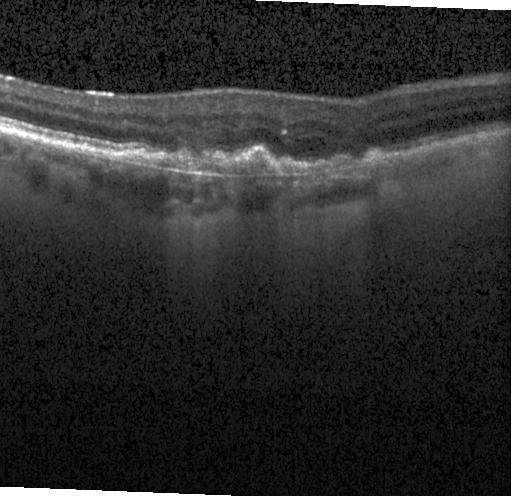

OCT line scan, spectral-domain optical coherence tomography, instrument: Heidelberg Spectralis. This B-scan demonstrates a choroidal neovascular membrane.